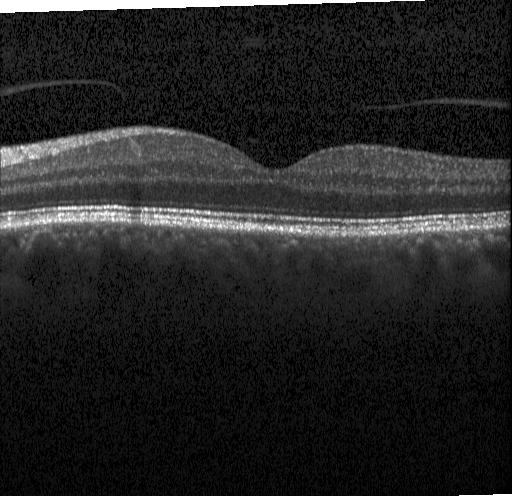

Macular scan, acquired on a Heidelberg Spectralis, spectral-domain optical coherence tomography, OCT B-scan. Finding: no choroidal neovascularization, no diabetic macular edema, and no drusen.